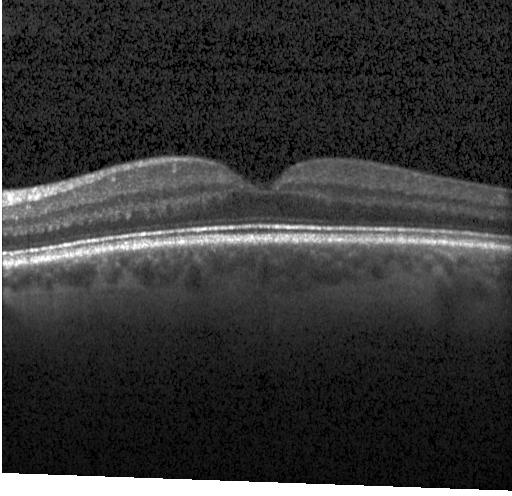

Optical coherence tomography scan
Dx: no evidence of CNV, DME, or drusen.